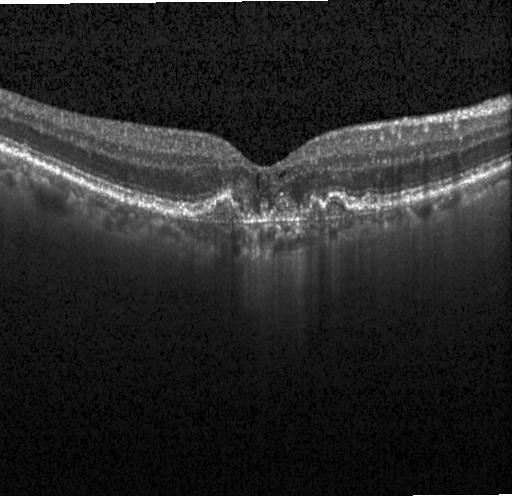
Optical coherence tomography B-scan, fovea-centered, spectral-domain OCT, acquired on a Heidelberg Spectralis — Finding: a choroidal neovascular membrane.